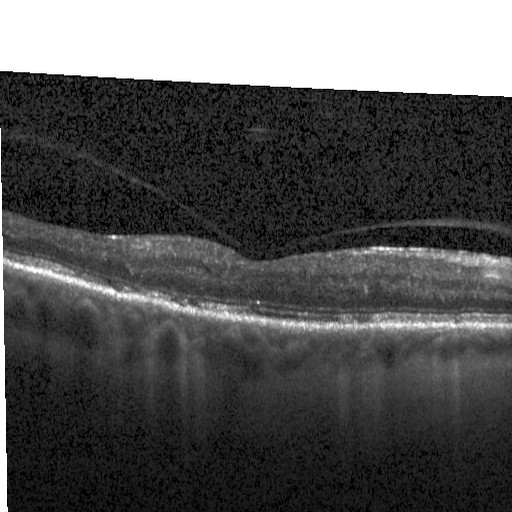
OCT scan showing DME.